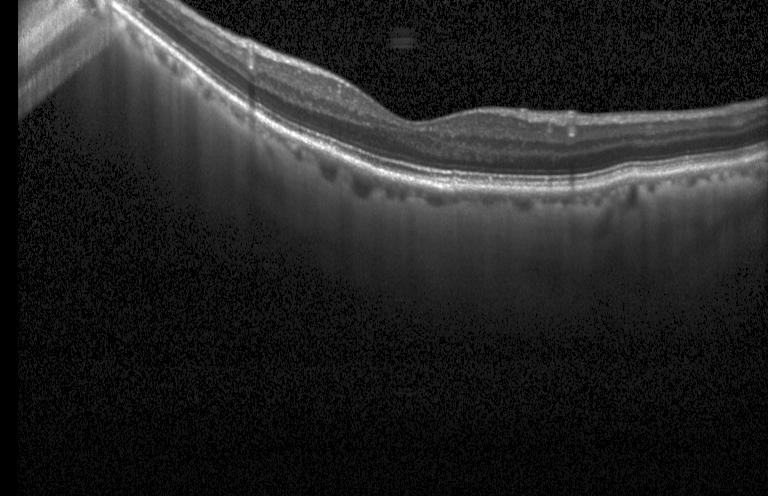

Retinal OCT cross-section.
Dx: no evidence of CNV, DME, or drusen.